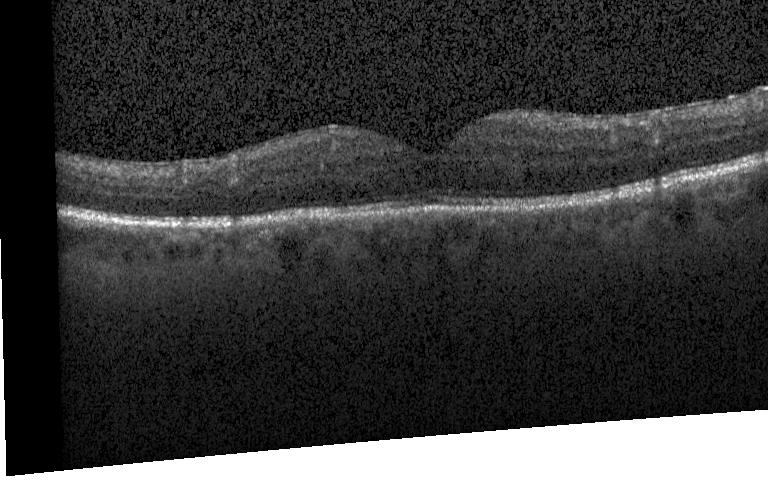

OCT B-scan. Spectral-domain OCT. Fovea-centered — Impression: no CNV, no DME, and no drusen.